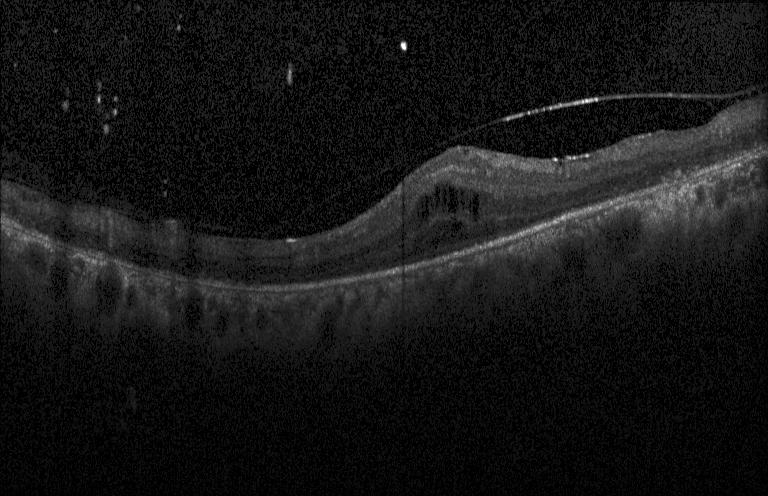

OCT finding: DME.